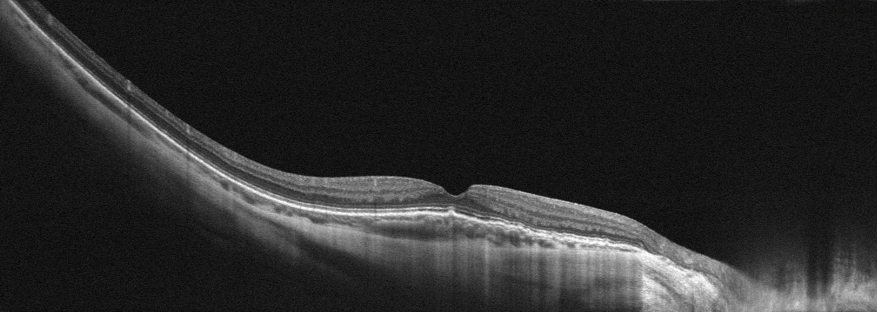 This B-scan demonstrates AMD.